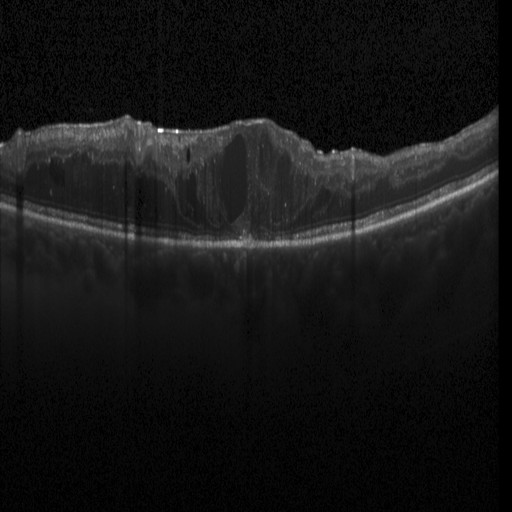 Impression: diabetic macular edema.